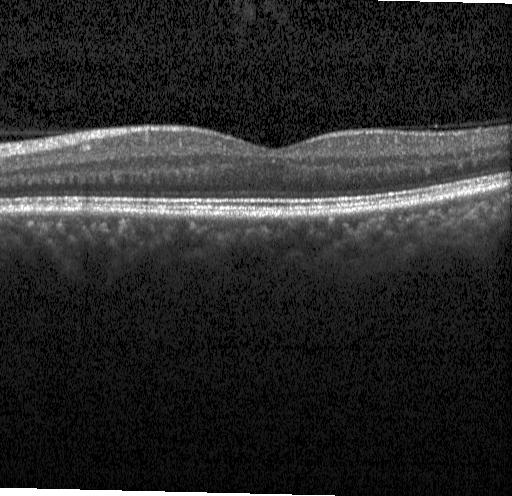

Spectral-domain optical coherence tomography, retinal OCT B-scan
Finding: neither choroidal neovascularization, diabetic macular edema, nor drusen.